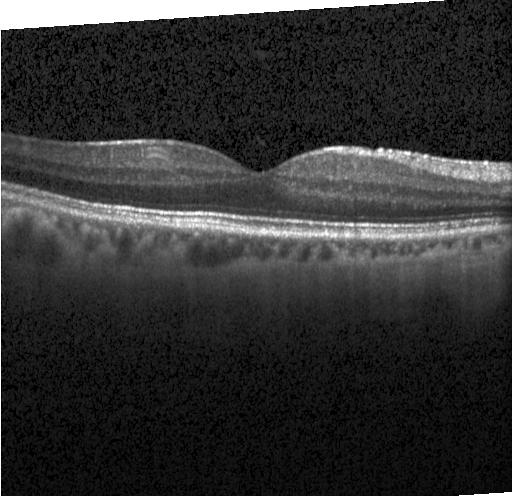
OCT line scan. Horizontal scan through the fovea. Neither choroidal neovascularization, diabetic macular edema, nor drusen.